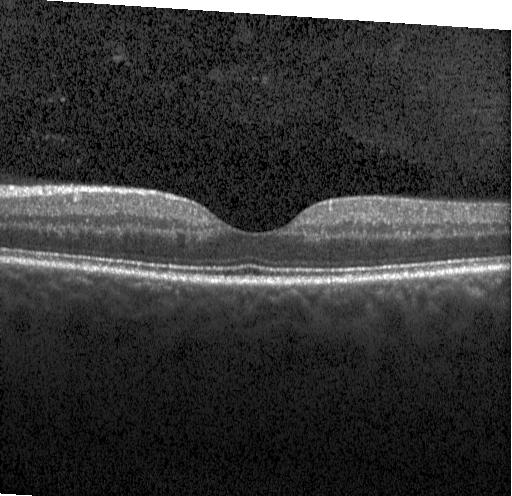 Optical coherence tomography scan, Heidelberg Spectralis. The scan shows neither CNV, DME, nor drusen.